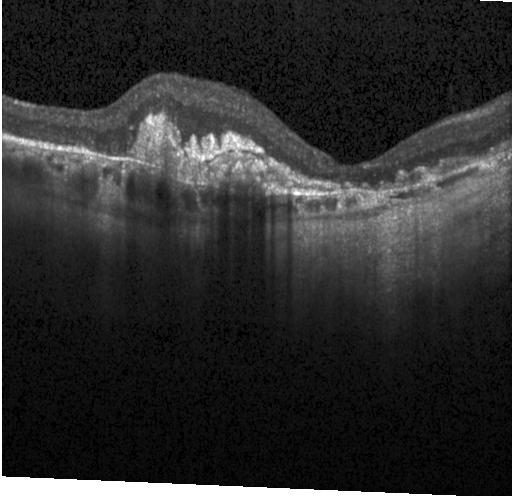

Heidelberg Spectralis OCT system. Retinal OCT cross-section — Diagnosis: CNV.